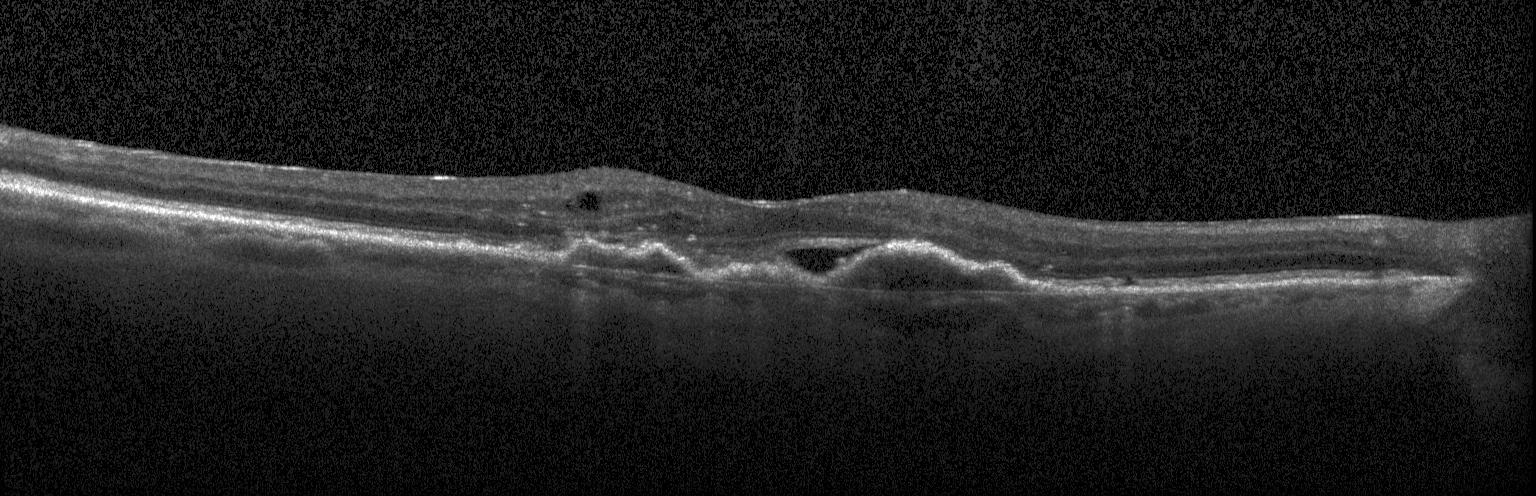

Assessment: CNV.